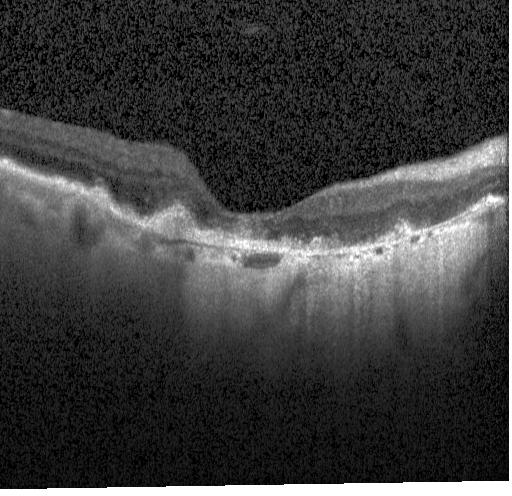

Through the macula; instrument: Heidelberg Spectralis; optical coherence tomography B-scan; spectral-domain optical coherence tomography
Diagnosis: a choroidal neovascular membrane.